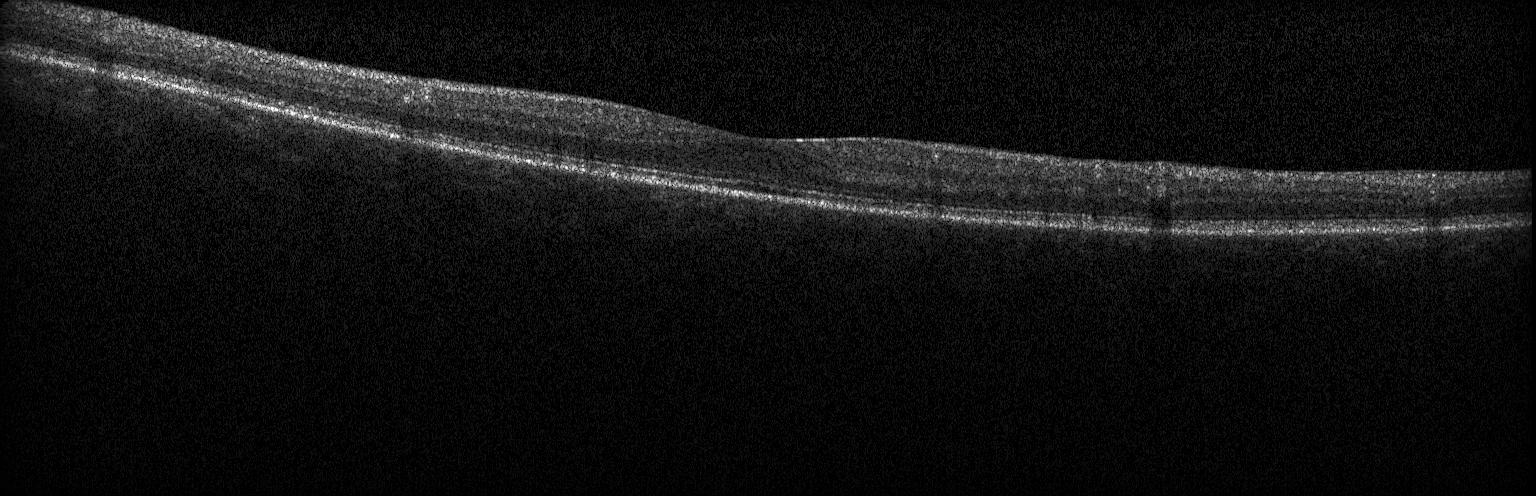 OCT B-scan — Diagnosis: no evidence of CNV, DME, or drusen.